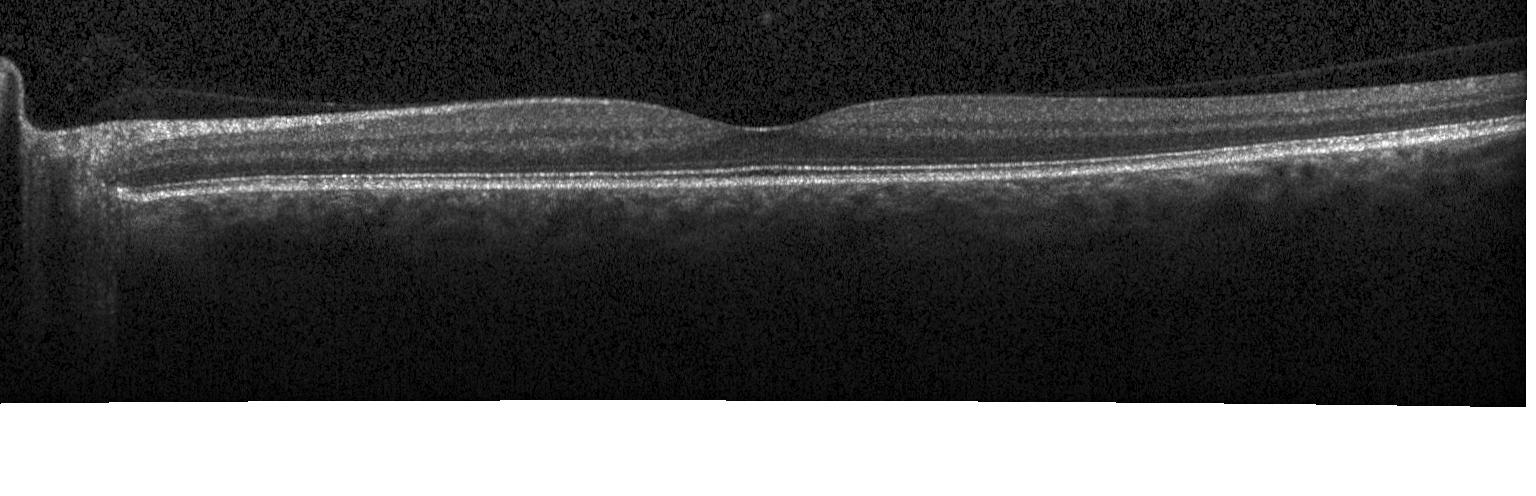 No evidence of CNV, DME, or drusen.